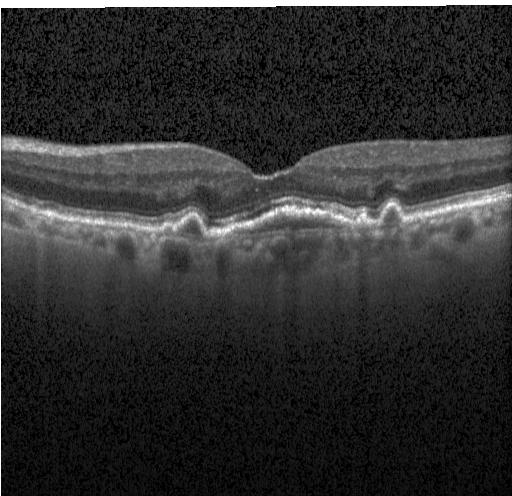
OCT B-scan — The scan shows choroidal neovascularization.